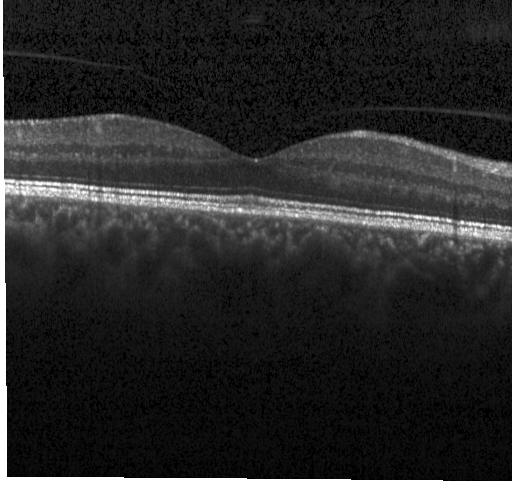

Dx: no choroidal neovascularization, no diabetic macular edema, and no drusen.